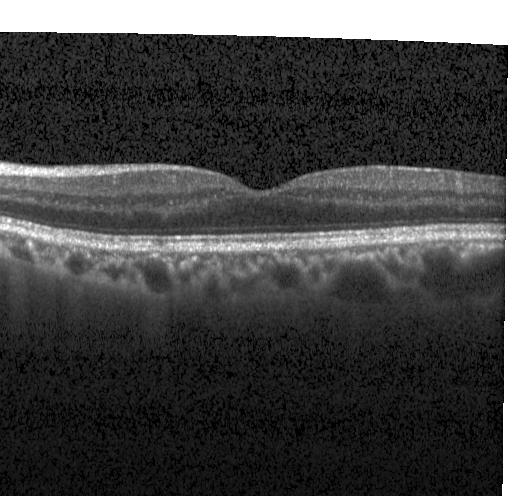
Retinal OCT cross-section
No evidence of choroidal neovascularization, diabetic macular edema, or drusen.